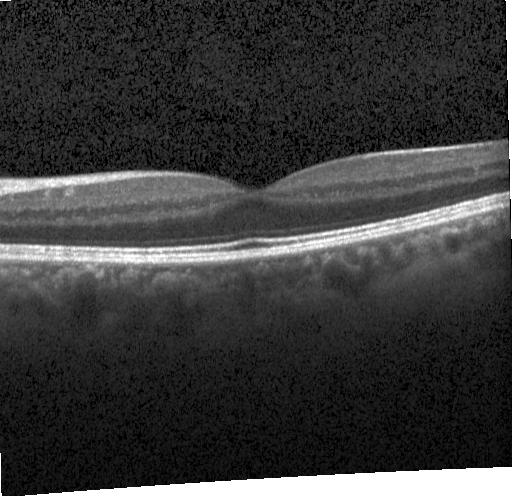

Spectral-domain OCT, OCT B-scan. Impression: no choroidal neovascularization, no diabetic macular edema, and no drusen.